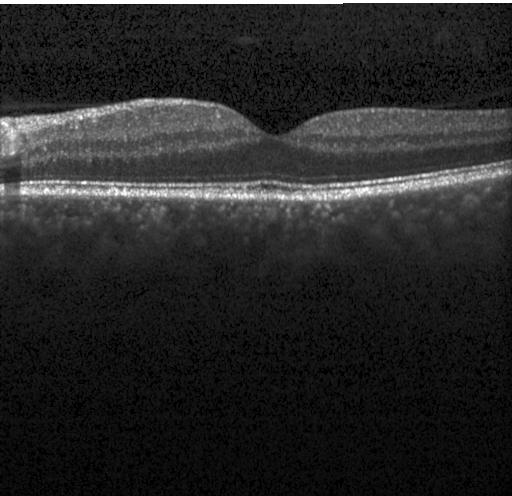 Optical coherence tomography scan — No choroidal neovascularization, diabetic macular edema, or drusen.